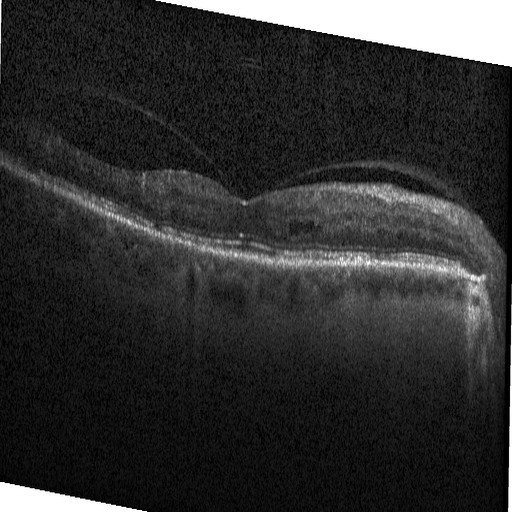
OCT B-scan showing DME.